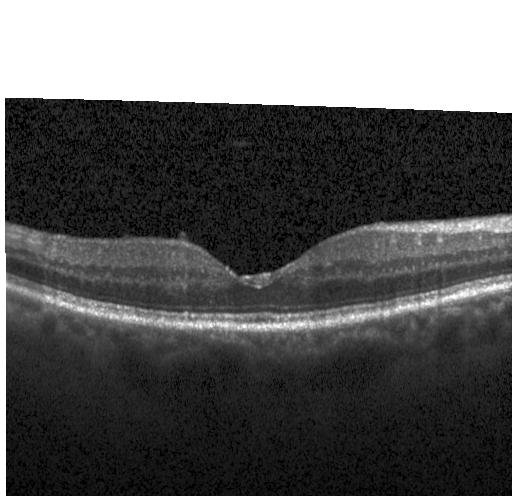

OCT line scan.
Impression: no CNV, no DME, and no drusen.